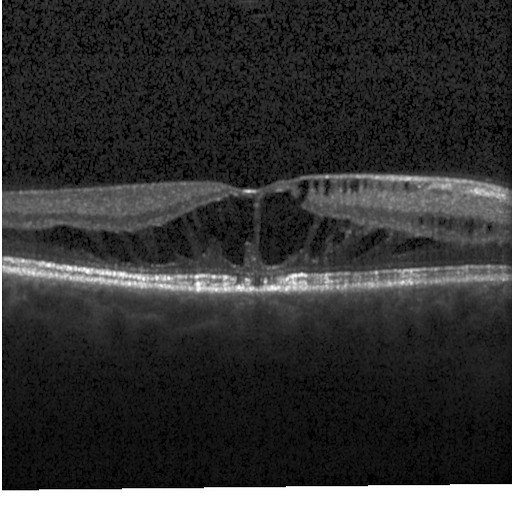 Centered on the fovea. Heidelberg Spectralis. Optical coherence tomography scan. Spectral-domain OCT
Assessment: diabetic macular edema (DME).